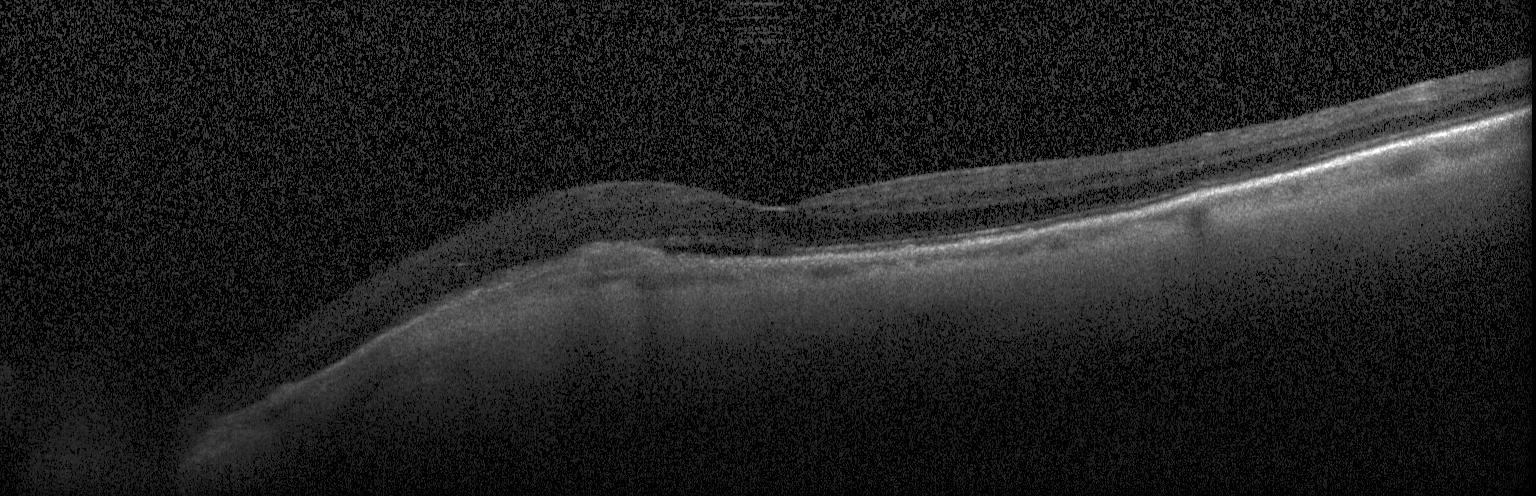
Macular OCT: choroidal neovascularization.